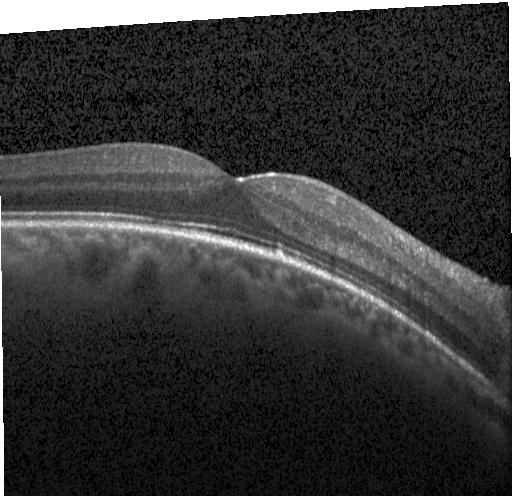

Dx: no choroidal neovascularization, diabetic macular edema, or drusen.